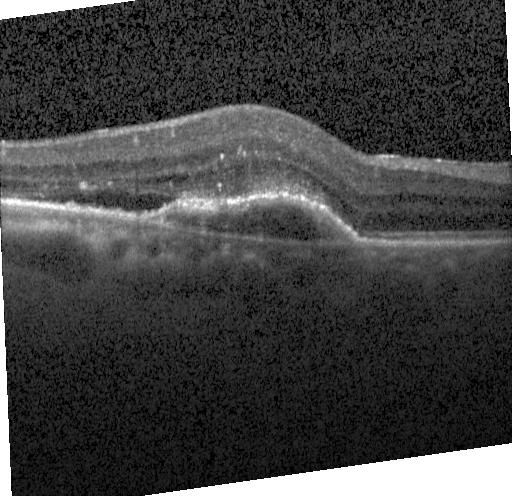 Finding: a choroidal neovascular membrane.